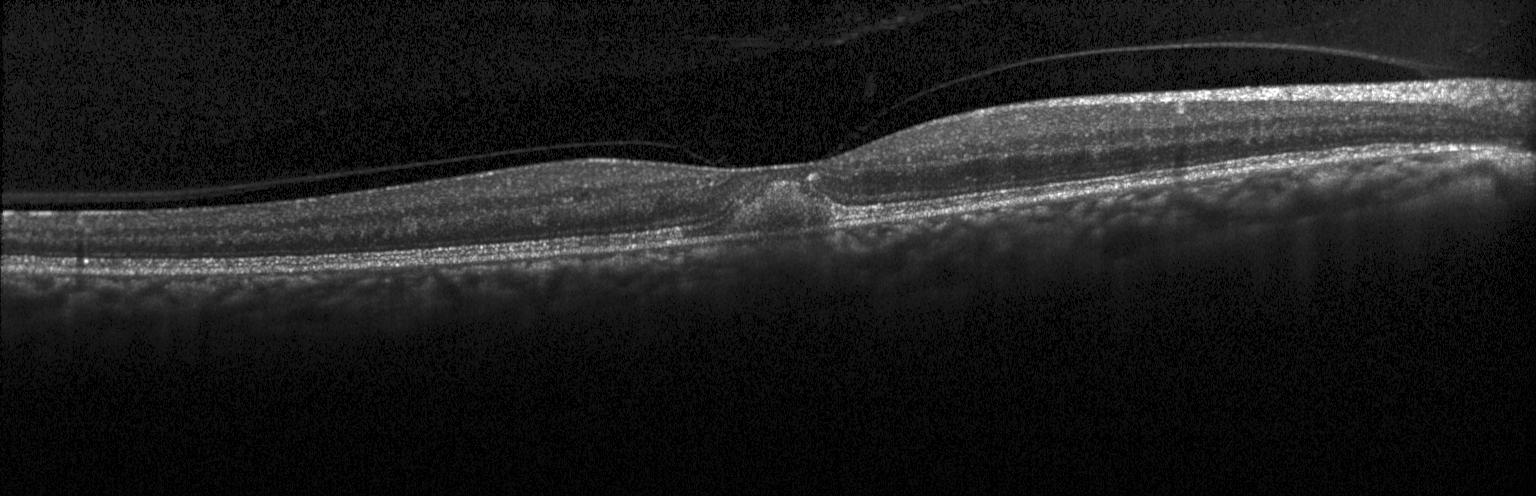
Dx: CNV.